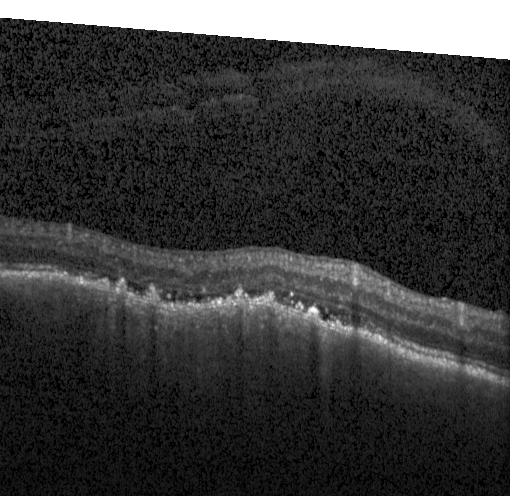
Spectral-domain optical coherence tomography, instrument: Heidelberg Spectralis, fovea-centered, optical coherence tomography scan.
Impression: a choroidal neovascular membrane.